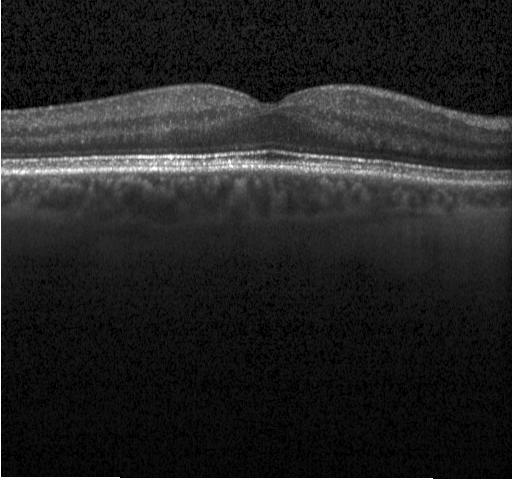
Retinal OCT cross-section showing no choroidal neovascularization, no diabetic macular edema, and no drusen.